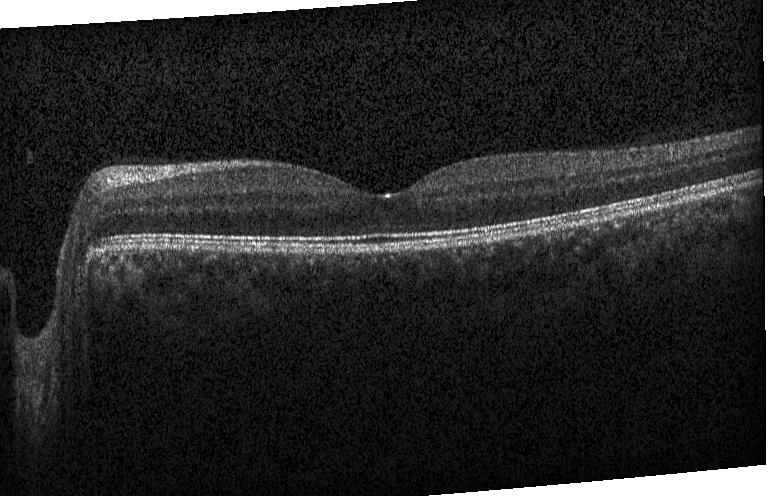
SD-OCT; fovea-centered; OCT B-scan; acquired on a Heidelberg Spectralis. Finding: neither choroidal neovascularization, diabetic macular edema, nor drusen.